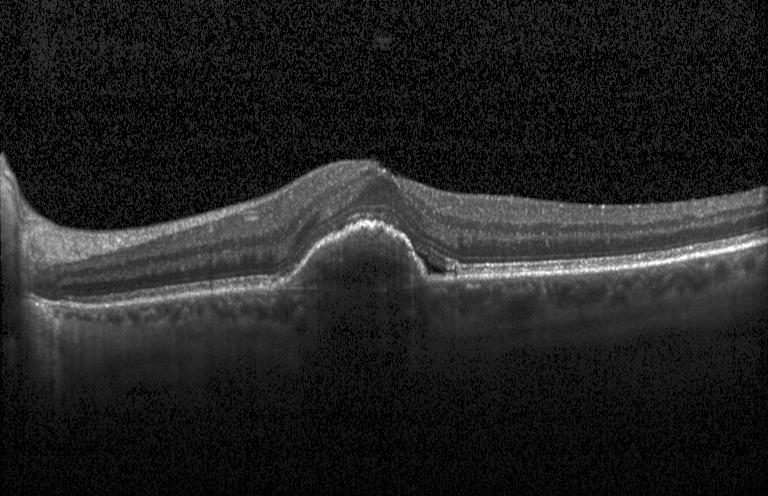

OCT finding: a choroidal neovascular membrane.